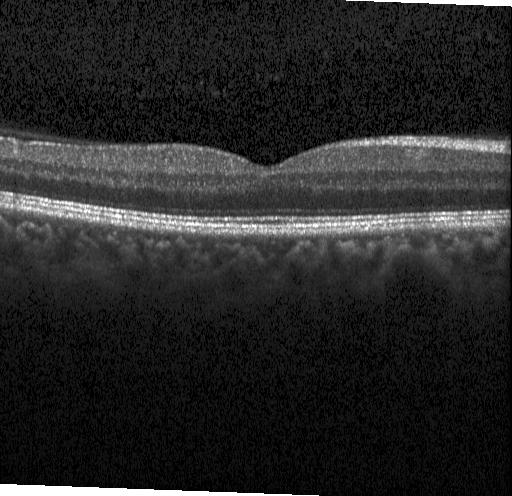

OCT B-scan showing neither CNV, DME, nor drusen.